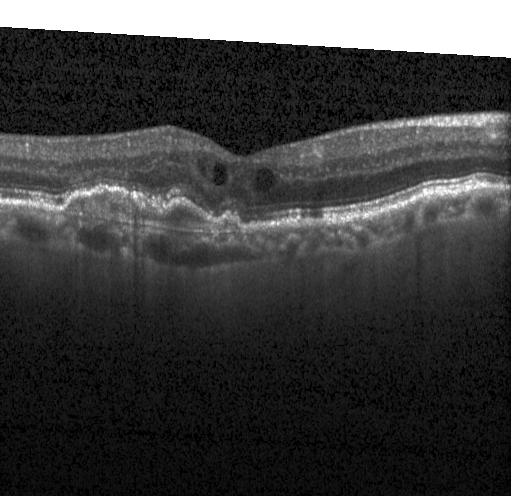 SD-OCT · OCT line scan.
This B-scan demonstrates choroidal neovascularization (CNV).